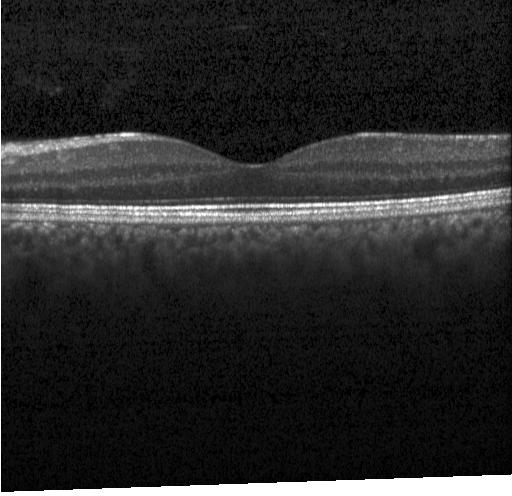

Retinal OCT cross-section — Assessment: no evidence of CNV, DME, or drusen.